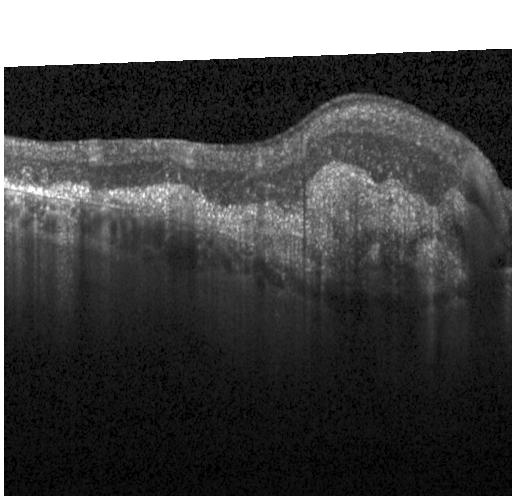 Retinal OCT B-scan · SD-OCT
OCT finding: a choroidal neovascular membrane.